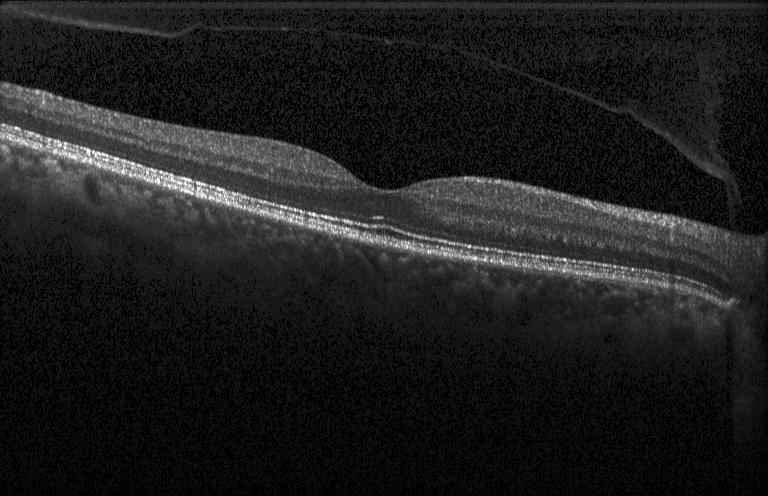 This B-scan demonstrates no choroidal neovascularization, diabetic macular edema, or drusen.